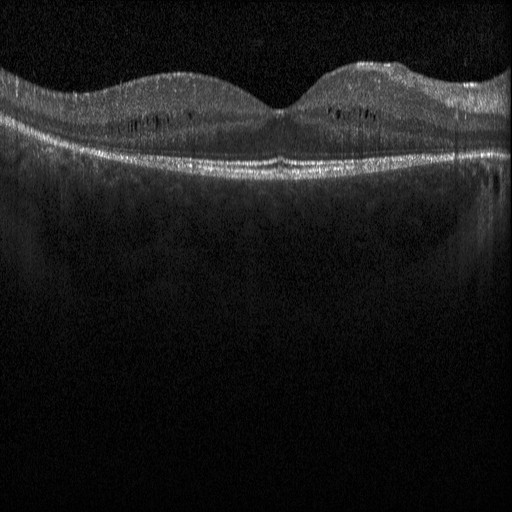
Acquired on a Heidelberg Spectralis · spectral-domain OCT · centered on the fovea · retinal OCT B-scan — OCT finding: diabetic macular edema.